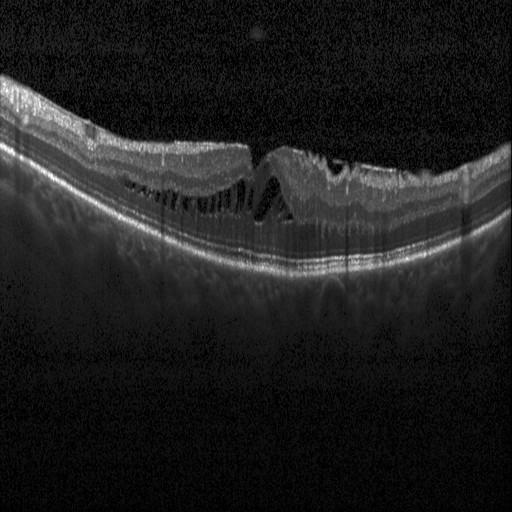

Macular OCT demonstrating diabetic macular edema.